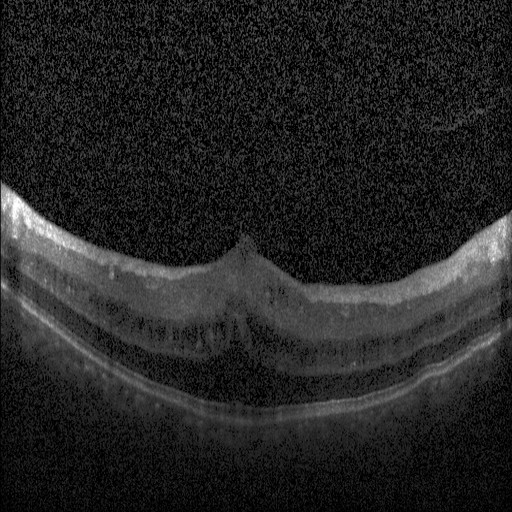

Heidelberg Spectralis; retinal OCT B-scan; centered on the fovea.
This B-scan demonstrates diabetic macular edema (DME).